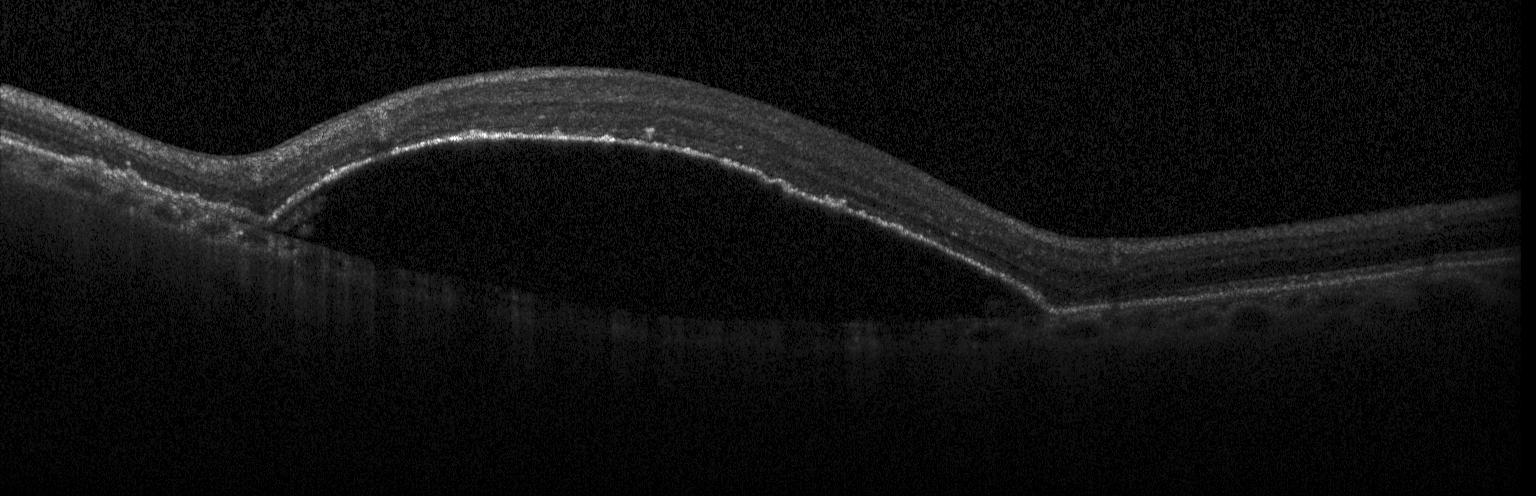
OCT scan showing CNV.